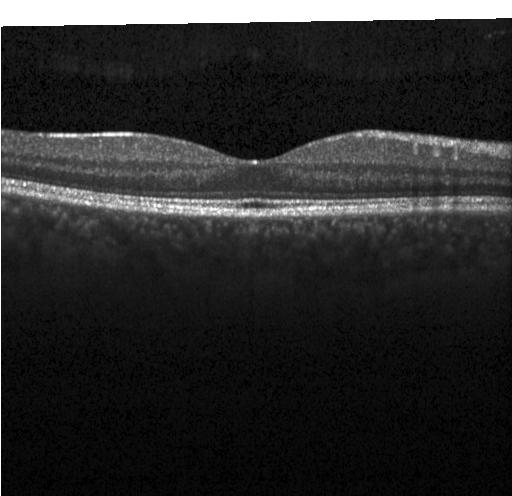

Fovea-centered, instrument: Heidelberg Spectralis, retinal OCT B-scan, SD-OCT. Impression: no evidence of choroidal neovascularization, diabetic macular edema, or drusen.